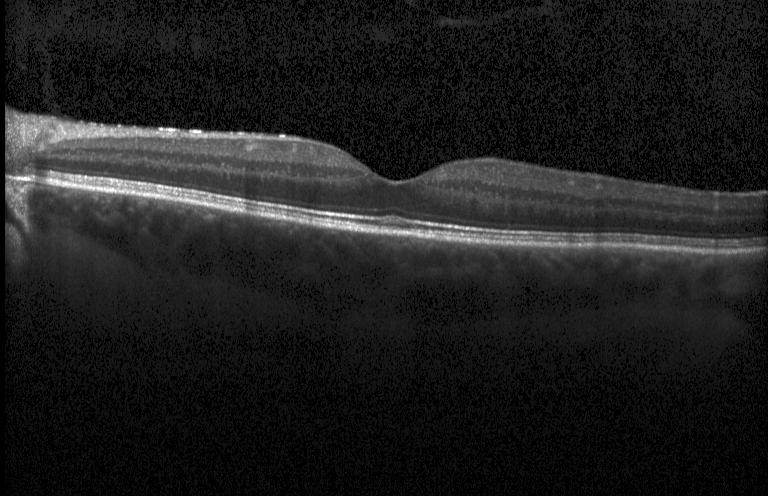

Impression: neither choroidal neovascularization, diabetic macular edema, nor drusen.